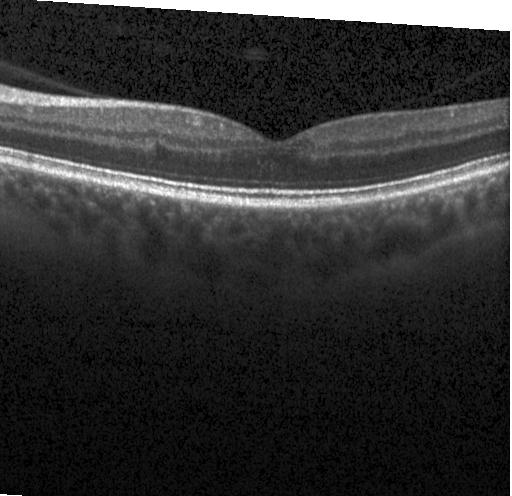 Optical coherence tomography scan · horizontal scan through the fovea
No choroidal neovascularization, no diabetic macular edema, and no drusen.